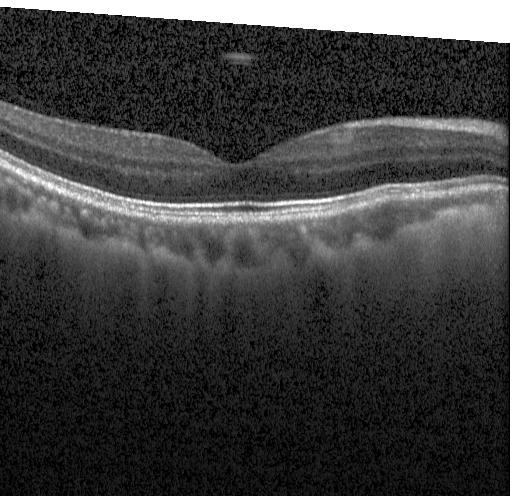
Assessment: no evidence of CNV, DME, or drusen.